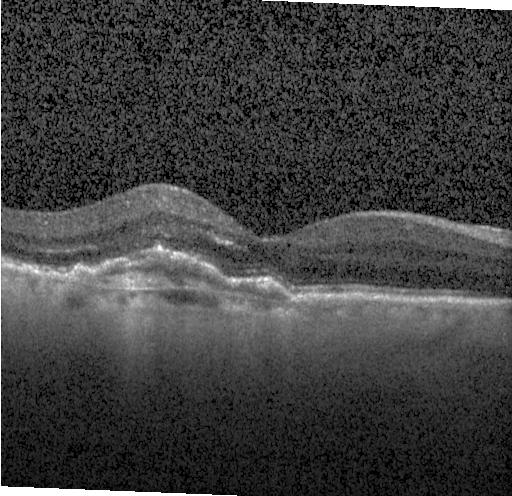
Optical coherence tomography B-scan
Finding: CNV.